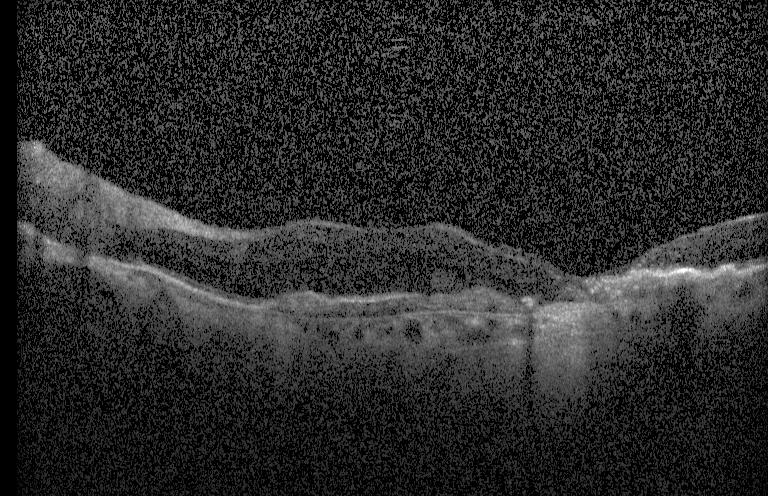 Retinal OCT cross-section, fovea-centered, Heidelberg Spectralis OCT system — Impression: choroidal neovascularization (CNV).